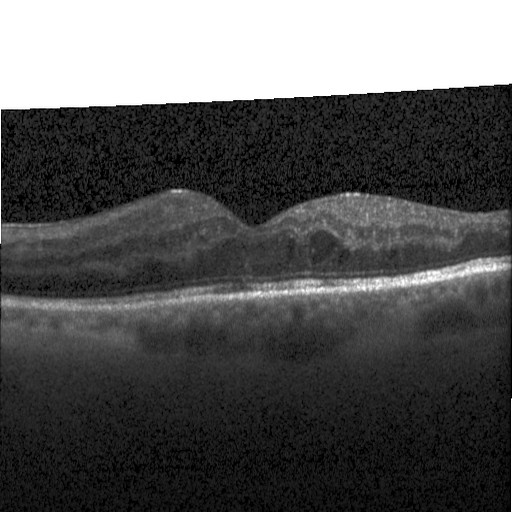
Assessment: diabetic macular edema.